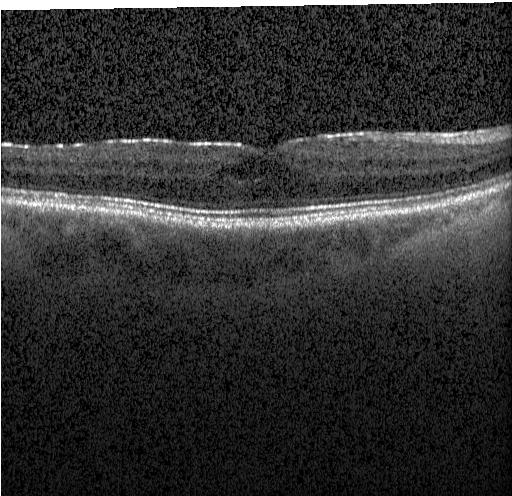 Retinal OCT B-scan
The scan shows DME.